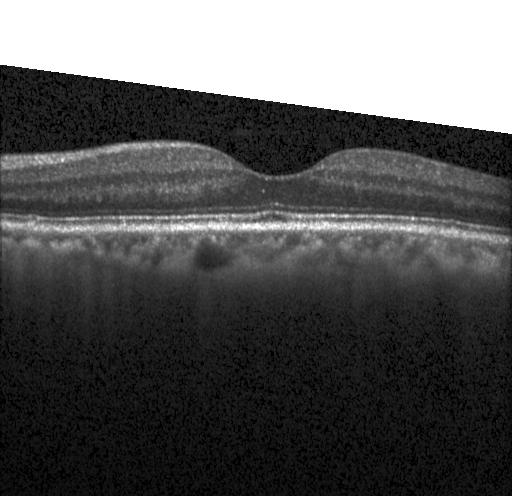 Retinal OCT cross-section. Dx: no CNV, DME, or drusen.